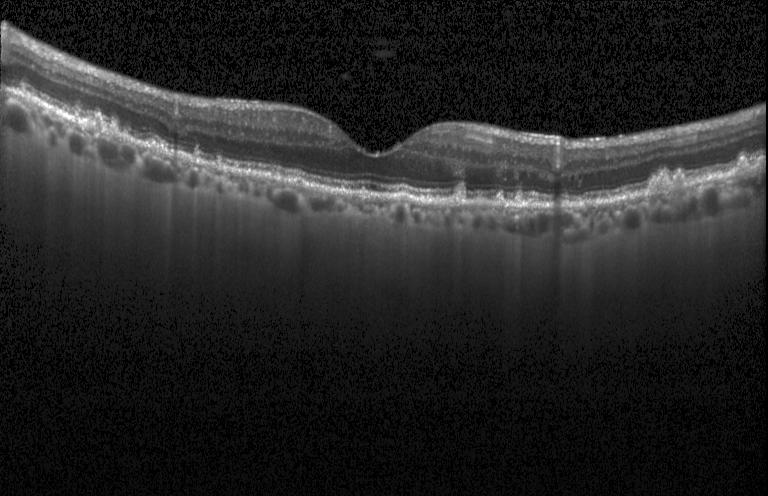
Optical coherence tomography B-scan · centered on the fovea. Impression: multiple drusen.